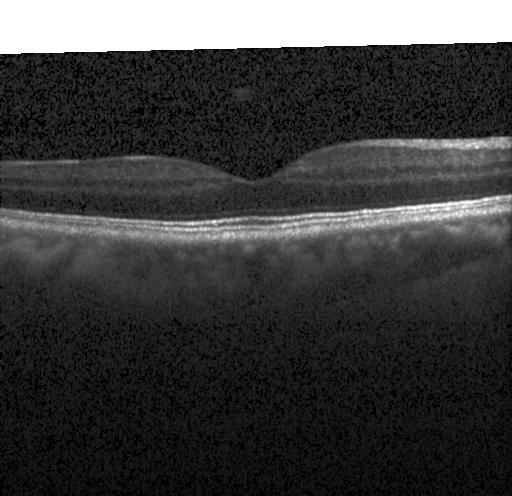

Retinal OCT cross-section. Finding: neither choroidal neovascularization, diabetic macular edema, nor drusen.